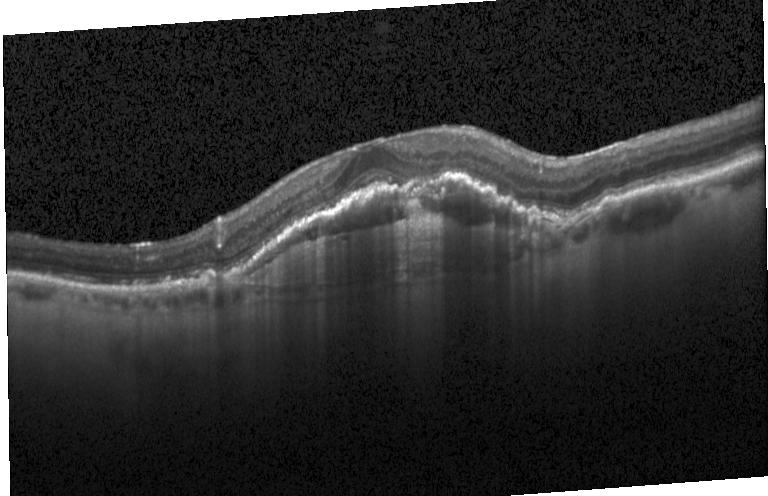

Finding: CNV.